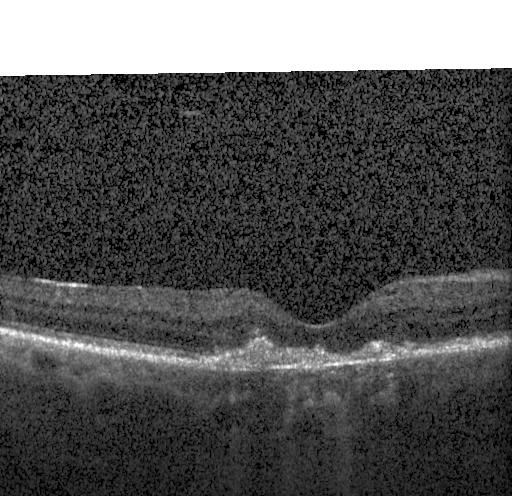
Macular OCT: choroidal neovascularization.